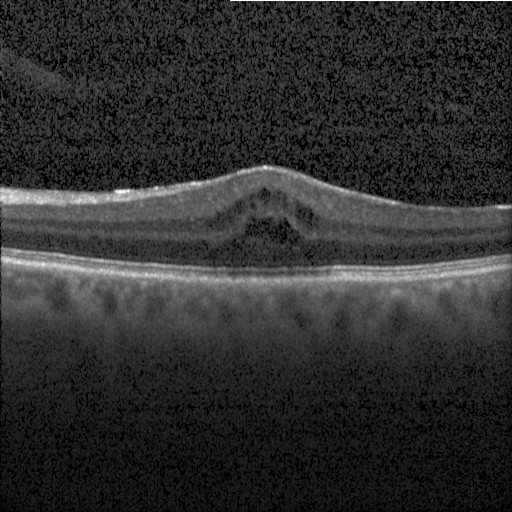
OCT scan showing diabetic macular edema (DME).